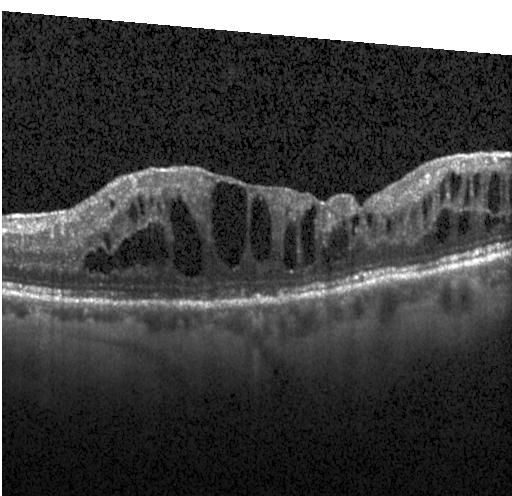 Through the macula; SD-OCT; acquired on a Heidelberg Spectralis; retinal OCT B-scan — Impression: diabetic macular edema (DME).